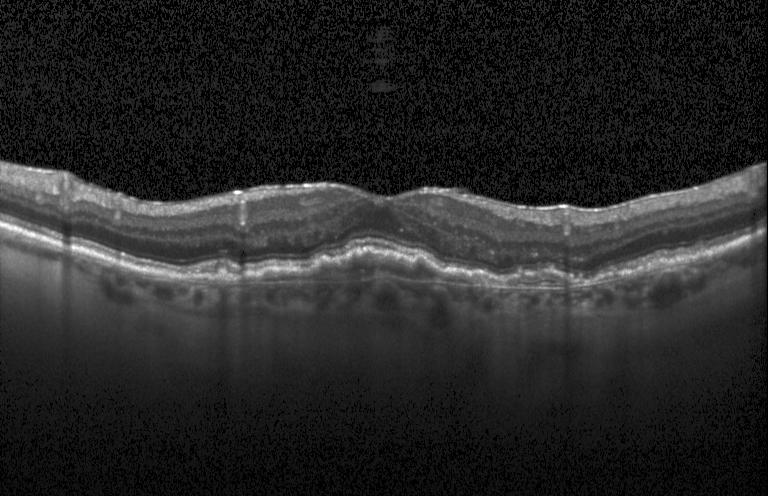 Macular scan; instrument: Heidelberg Spectralis; OCT B-scan; spectral-domain optical coherence tomography.
Diagnosis: CNV.